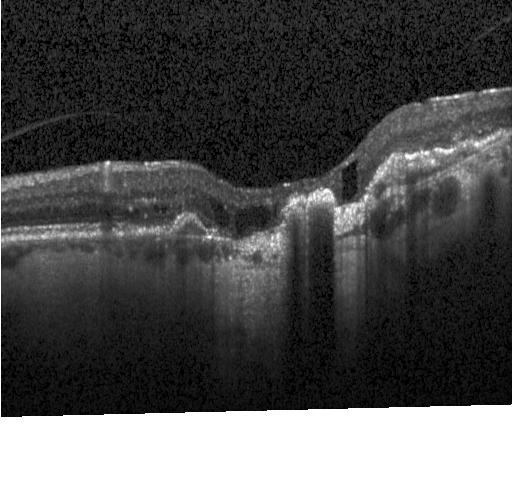

Spectral-domain optical coherence tomography, optical coherence tomography B-scan, Heidelberg Spectralis OCT system, through the macula.
Diagnosis: a choroidal neovascular membrane.